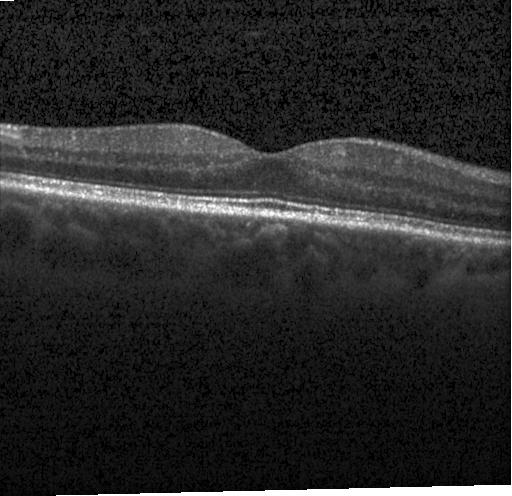

Retinal OCT cross-section — OCT finding: no evidence of choroidal neovascularization, diabetic macular edema, or drusen.